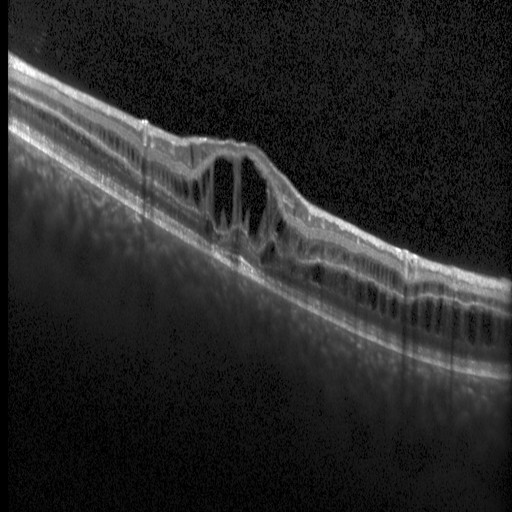

Heidelberg Spectralis OCT system · spectral-domain OCT · OCT B-scan · horizontal scan through the fovea — Assessment: diabetic macular edema.